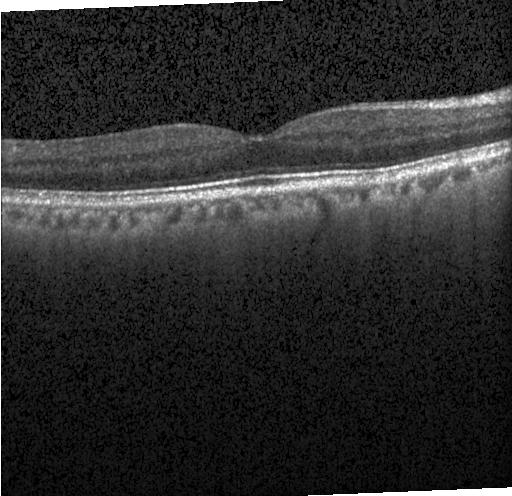 The scan shows no evidence of CNV, DME, or drusen.